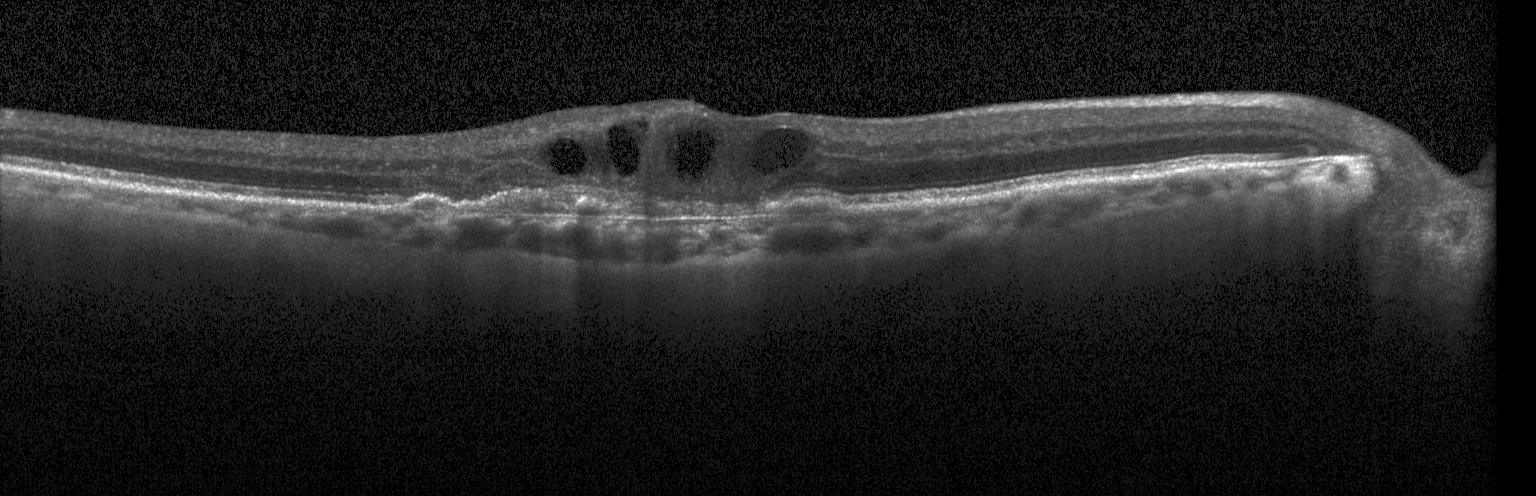
OCT finding: choroidal neovascularization (CNV).